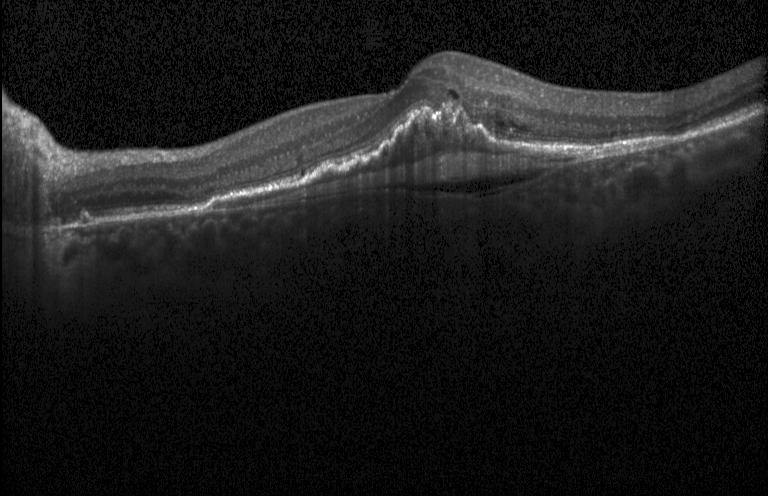 Impression: CNV.